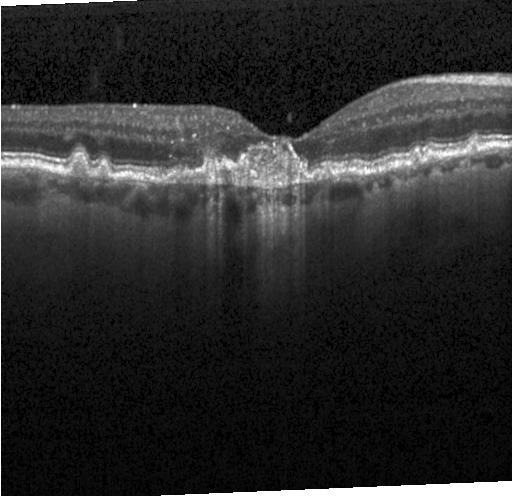
Retinal OCT B-scan; macular scan — Impression: a choroidal neovascular membrane.